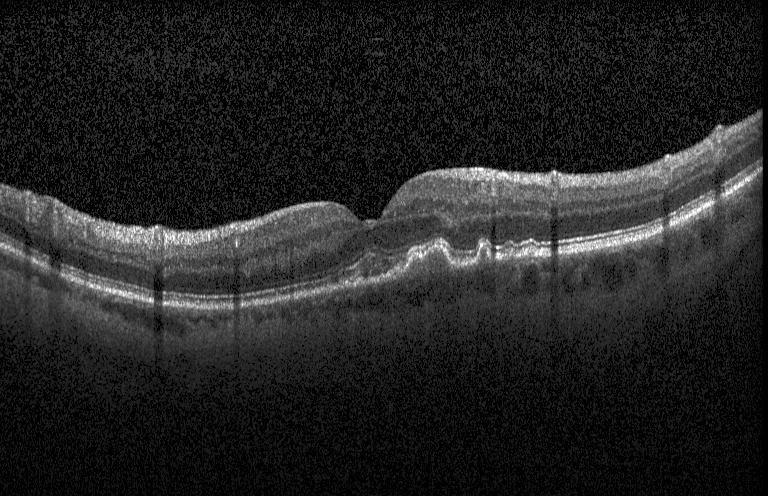 Macular OCT: drusen.